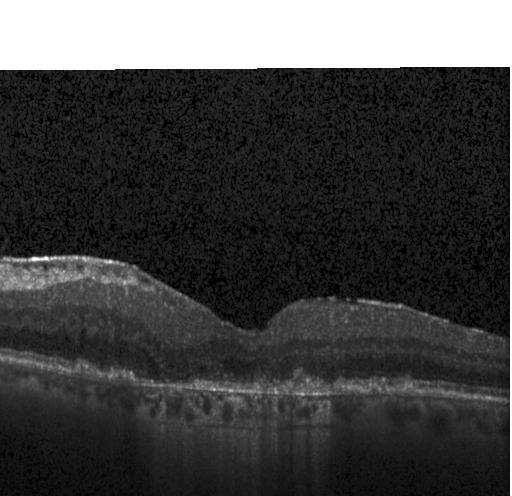 Heidelberg Spectralis OCT system. Optical coherence tomography scan. Spectral-domain OCT. Centered on the fovea. Macular OCT: a choroidal neovascular membrane.